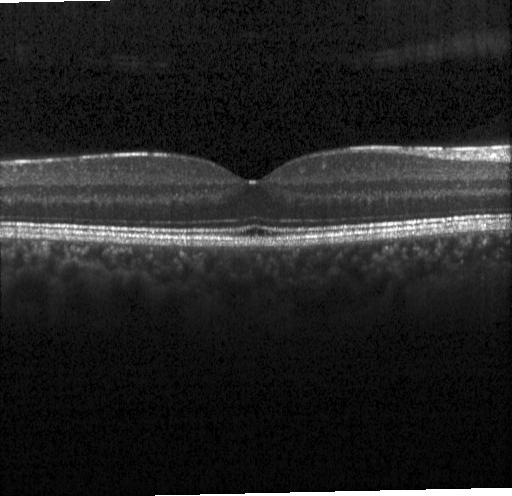 OCT line scan, spectral-domain optical coherence tomography
Diagnosis: neither choroidal neovascularization, diabetic macular edema, nor drusen.